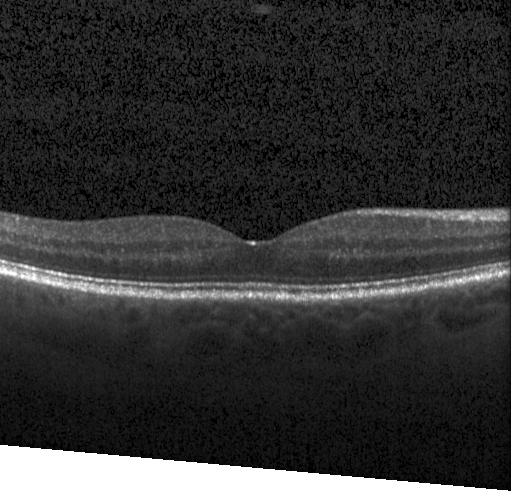 Optical coherence tomography scan
Diagnosis: no choroidal neovascularization, diabetic macular edema, or drusen.